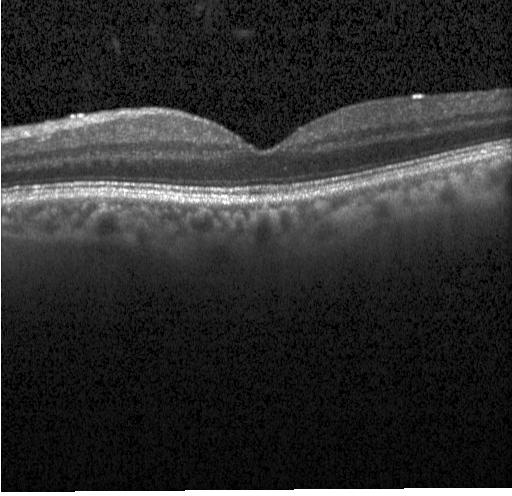

Retinal OCT cross-section showing no choroidal neovascularization, diabetic macular edema, or drusen.